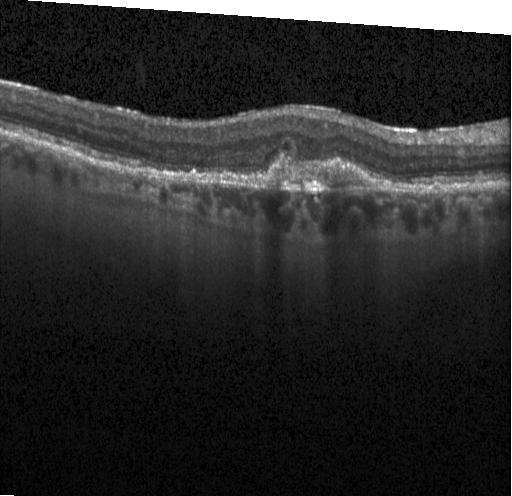
Macular OCT: CNV.